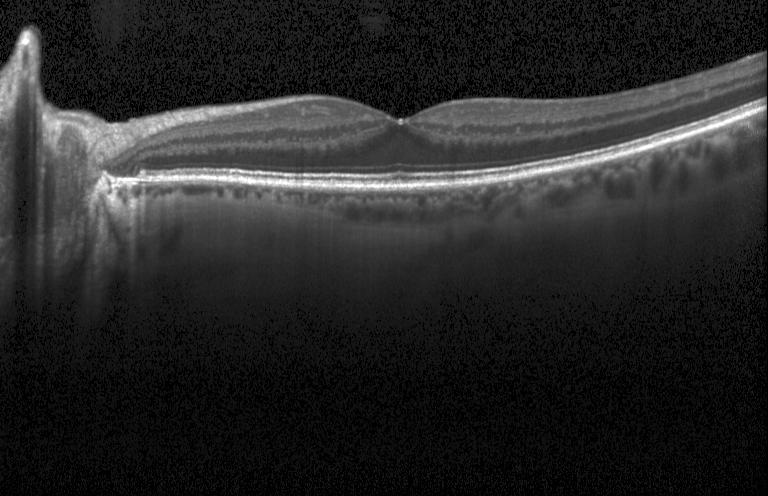

Macular OCT: neither choroidal neovascularization, diabetic macular edema, nor drusen.